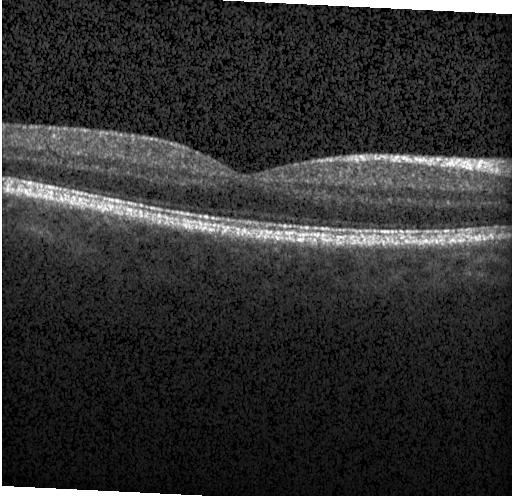
Dx: neither CNV, DME, nor drusen.